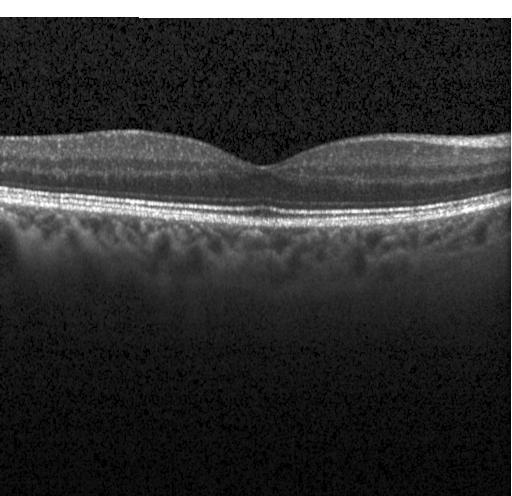
Finding: no choroidal neovascularization, diabetic macular edema, or drusen.